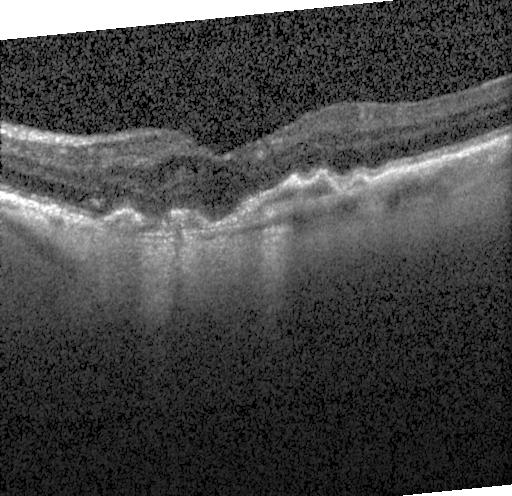
A choroidal neovascular membrane.